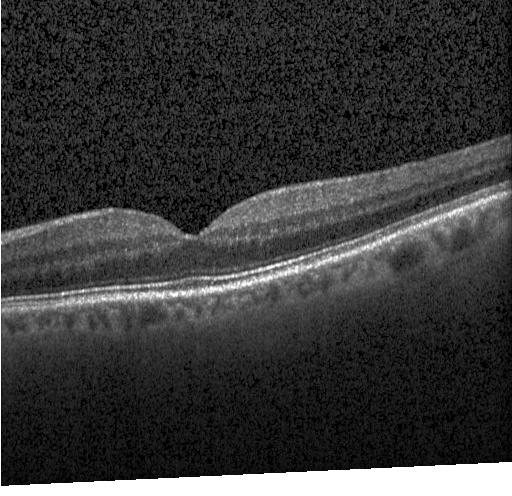 OCT B-scan · Heidelberg Spectralis · spectral-domain optical coherence tomography. Neither CNV, DME, nor drusen.